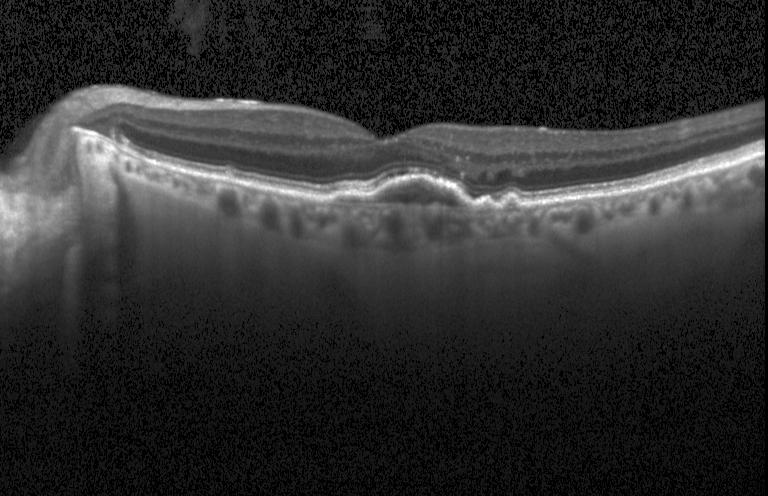

Instrument: Heidelberg Spectralis, optical coherence tomography scan, macular scan.
Impression: a choroidal neovascular membrane.